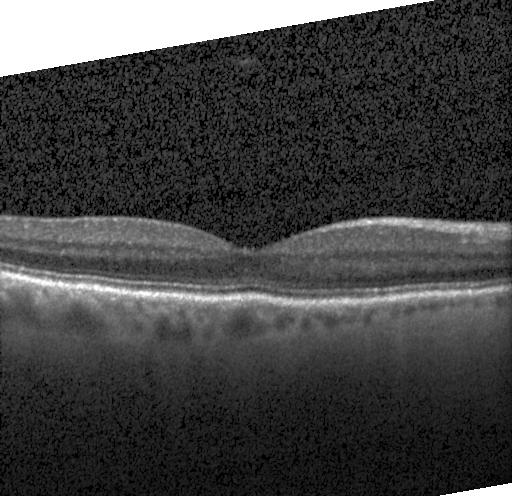

Horizontal scan through the fovea; Heidelberg Spectralis OCT system; optical coherence tomography B-scan; spectral-domain optical coherence tomography — Finding: no CNV, no DME, and no drusen.